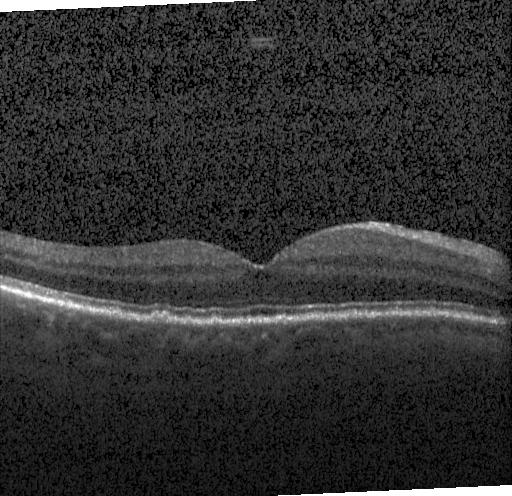 Optical coherence tomography scan, spectral-domain optical coherence tomography, macular scan.
OCT finding: sub-RPE drusenoid deposits.